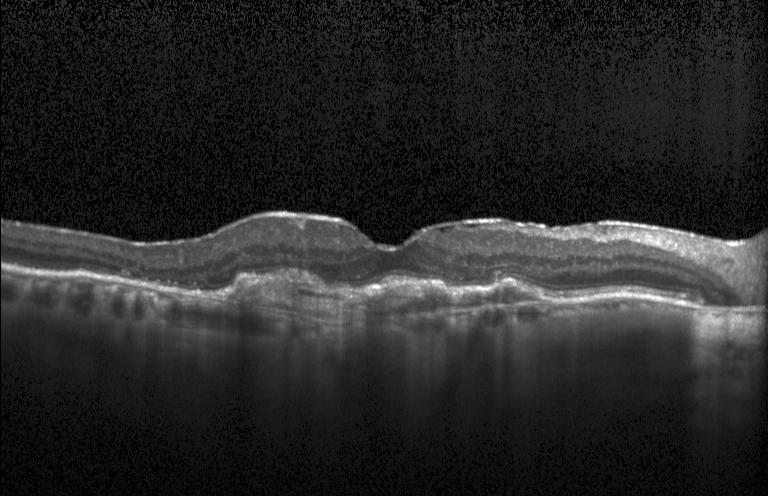 OCT finding: a choroidal neovascular membrane.